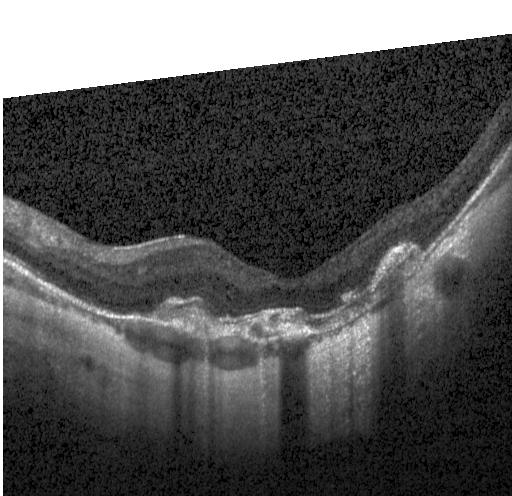 Retinal OCT B-scan — CNV.